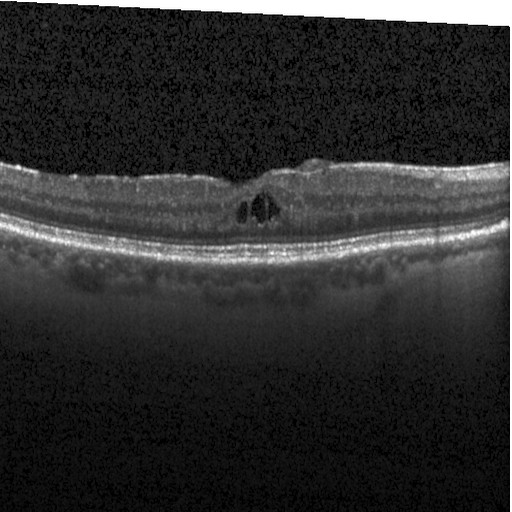
Spectral-domain optical coherence tomography, optical coherence tomography B-scan, through the macula — Finding: diabetic macular edema (DME).